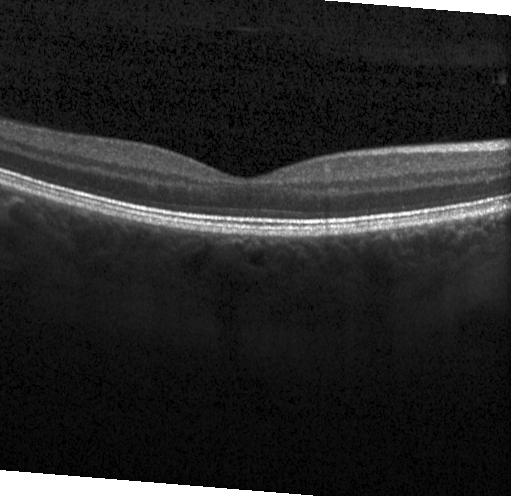
Retinal OCT cross-section showing no CNV, no DME, and no drusen.